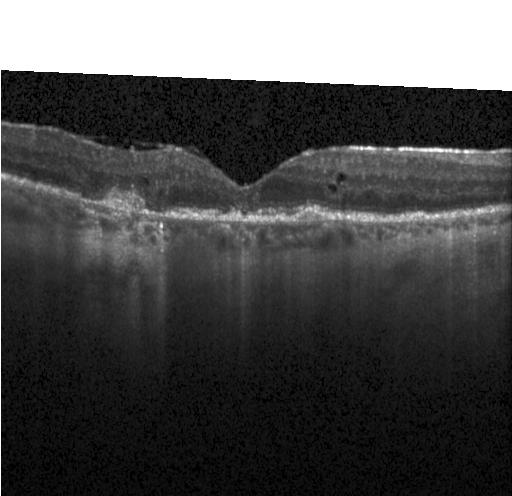 Horizontal scan through the fovea. Retinal OCT cross-section. Instrument: Heidelberg Spectralis. Spectral-domain optical coherence tomography — Assessment: CNV.